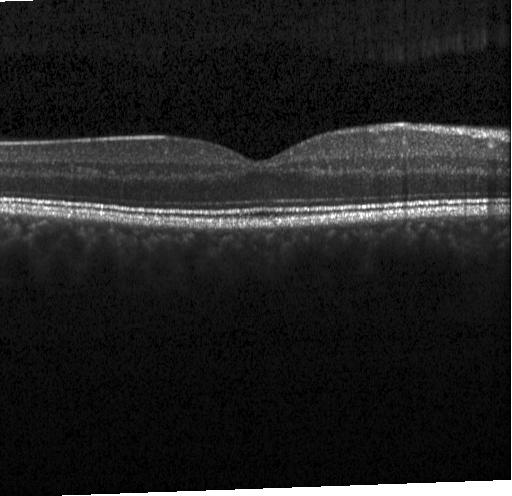 Retinal OCT B-scan — Assessment: no CNV, no DME, and no drusen.